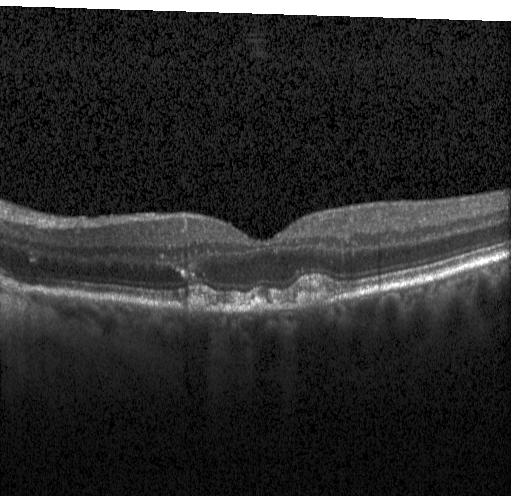 Retinal OCT B-scan; centered on the fovea; Heidelberg Spectralis; spectral-domain OCT
Diagnosis: sub-RPE drusenoid deposits.